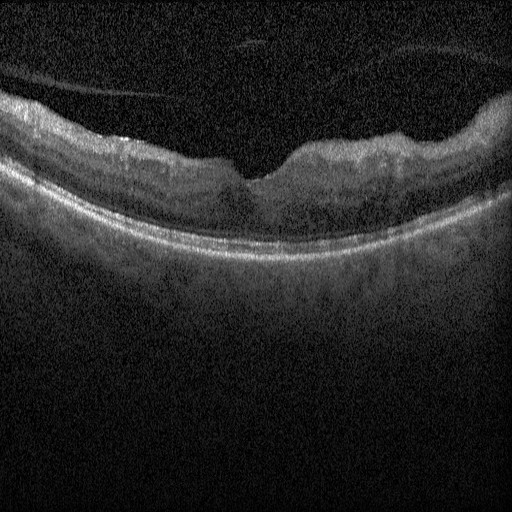

OCT B-scan. This B-scan demonstrates DME.